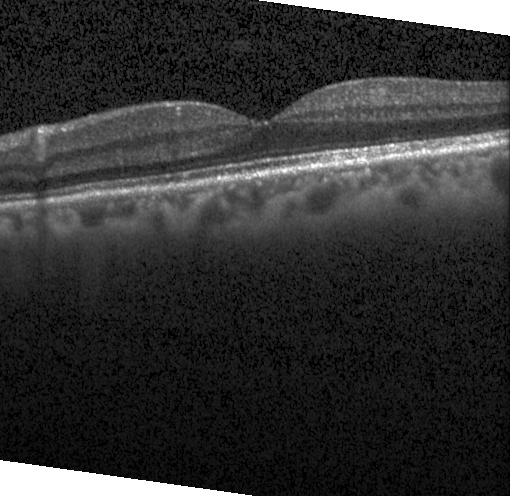

OCT finding: no evidence of choroidal neovascularization, diabetic macular edema, or drusen.